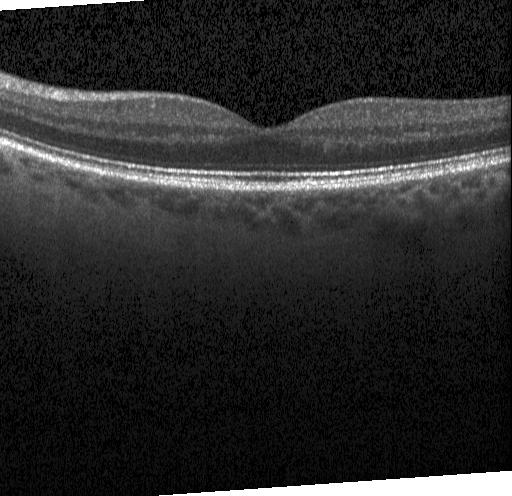

Optical coherence tomography B-scan
Finding: no CNV, DME, or drusen.